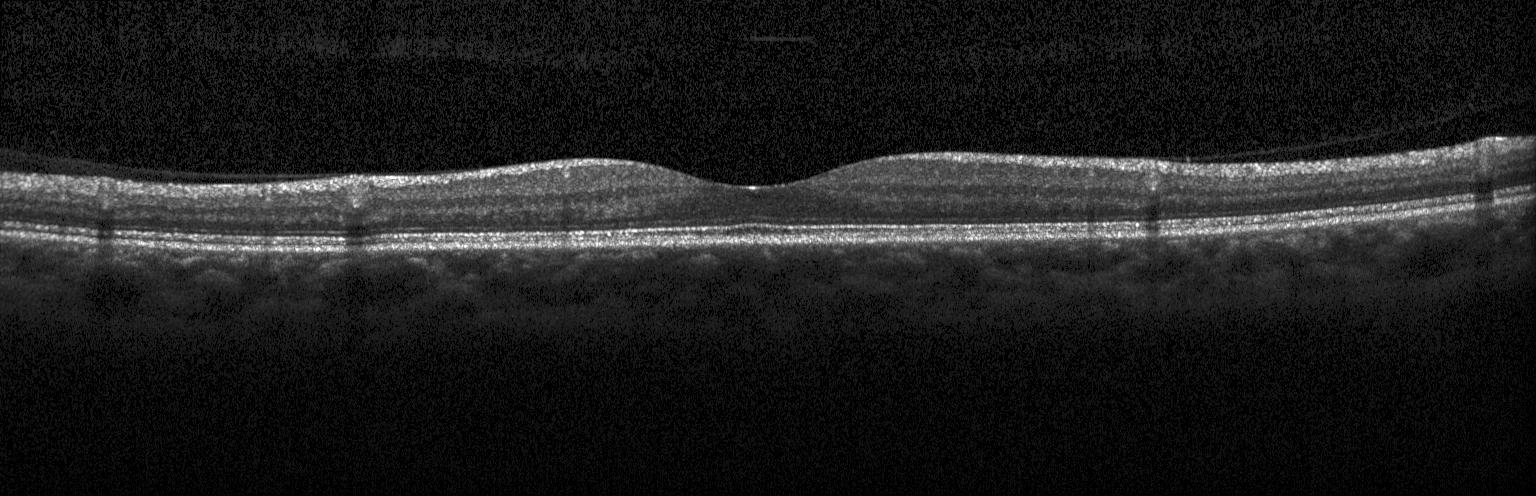
OCT B-scan · through the macula. OCT finding: no evidence of CNV, DME, or drusen.